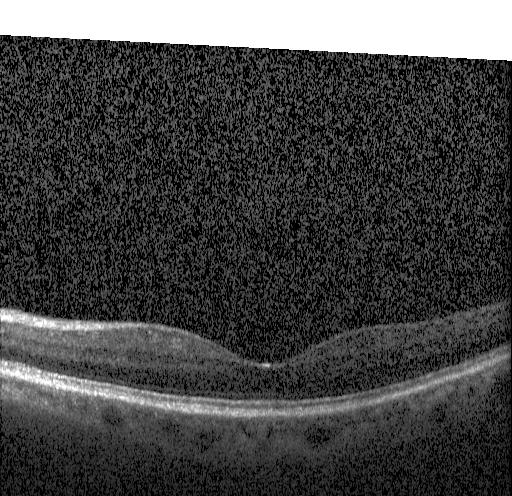 Macular OCT demonstrating no evidence of choroidal neovascularization, diabetic macular edema, or drusen.